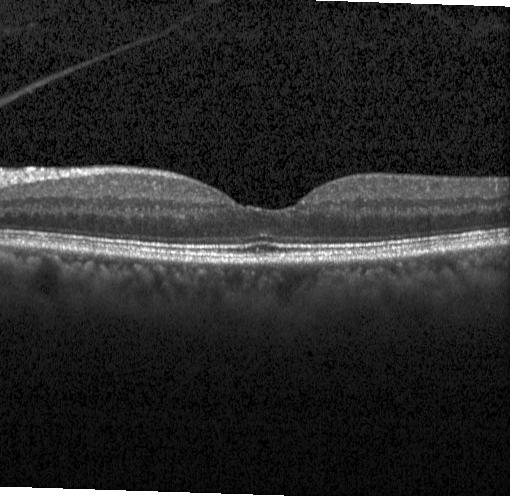 The scan shows no choroidal neovascularization, no diabetic macular edema, and no drusen.